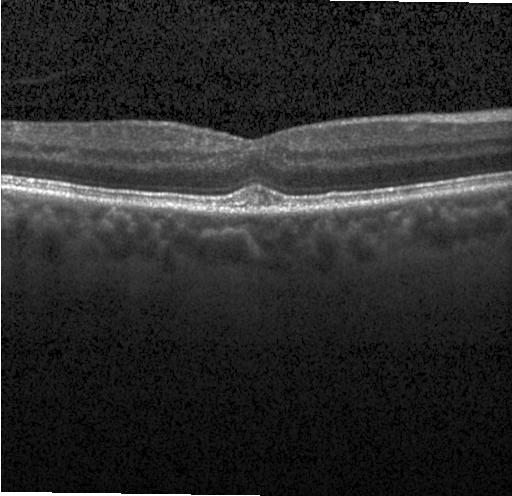

Optical coherence tomography B-scan, spectral-domain OCT, Heidelberg Spectralis — Sub-RPE drusenoid deposits.